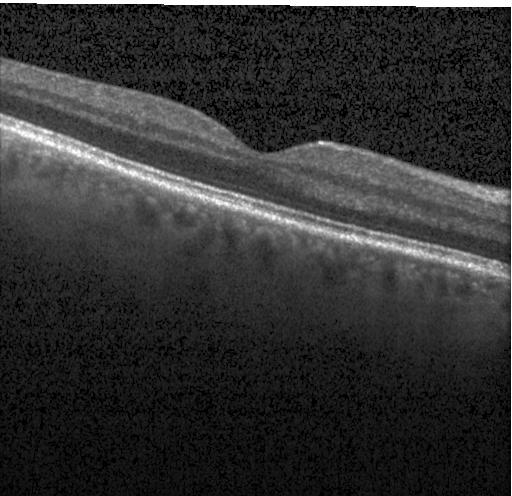
Retinal OCT B-scan, Heidelberg Spectralis OCT system, macular scan, SD-OCT — Impression: no choroidal neovascularization, diabetic macular edema, or drusen.